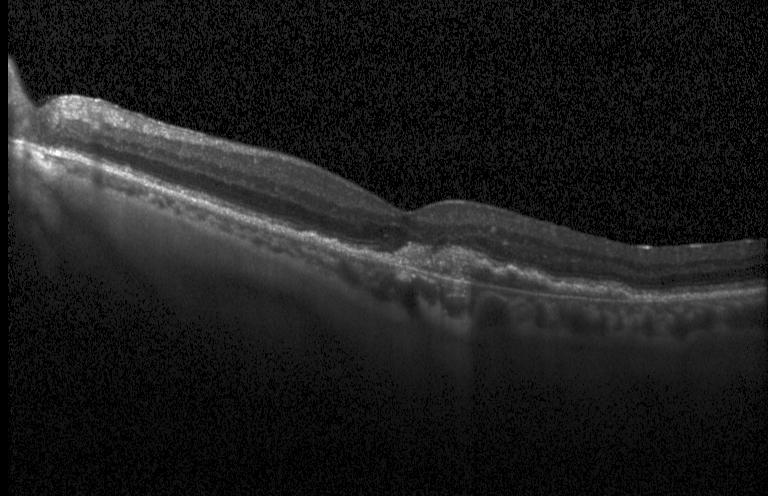 OCT B-scan showing choroidal neovascularization.